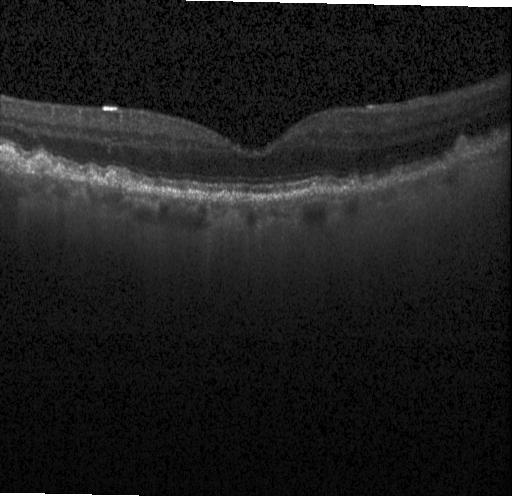 Spectral-domain OCT B-scan: multiple drusen.